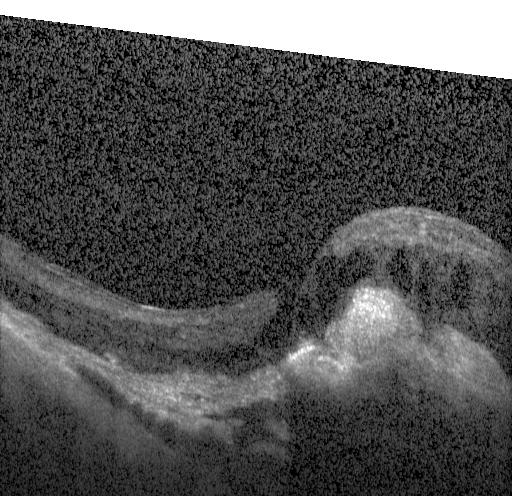 Macular scan. Retinal OCT cross-section. Spectral-domain optical coherence tomography. Diagnosis: a choroidal neovascular membrane.